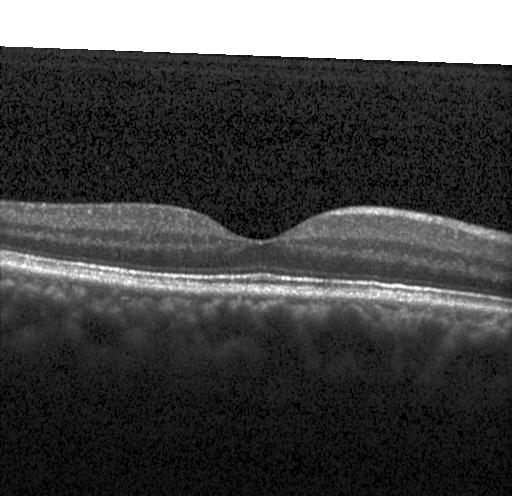

Optical coherence tomography scan — Diagnosis: no CNV, no DME, and no drusen.